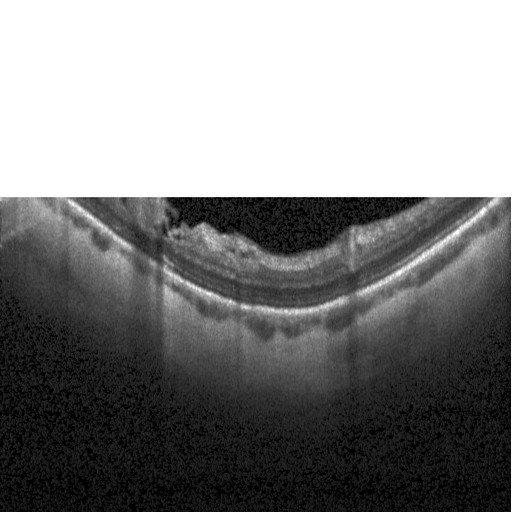

OCT line scan. Diagnosis: diabetic macular edema (DME).